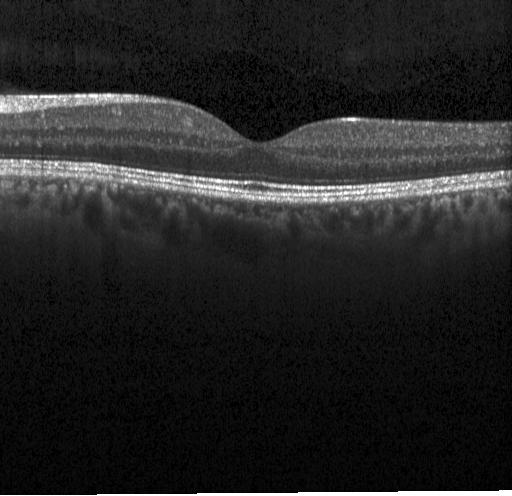

OCT B-scan — No evidence of CNV, DME, or drusen.